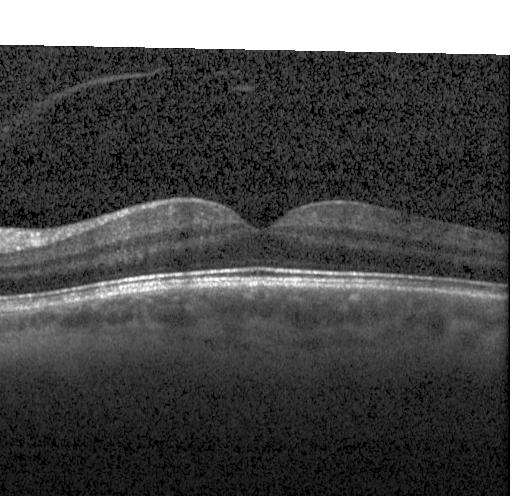 SD-OCT · acquired on a Heidelberg Spectralis · through the macula · retinal OCT cross-section
Impression: neither CNV, DME, nor drusen.